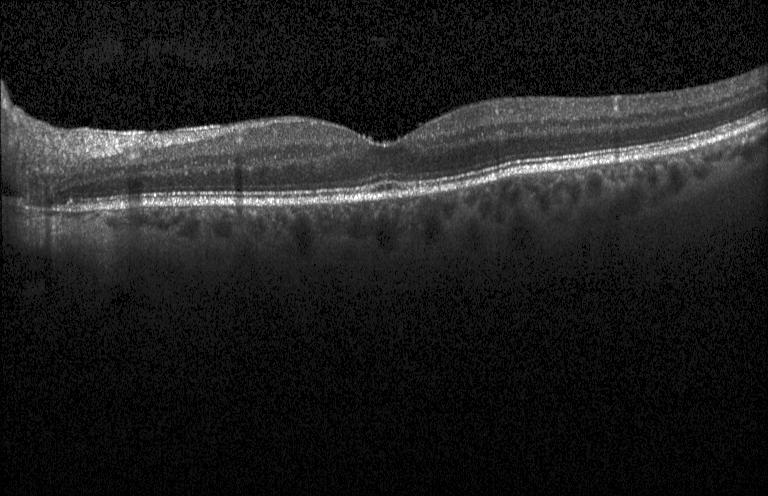

OCT B-scan; spectral-domain optical coherence tomography — No choroidal neovascularization, diabetic macular edema, or drusen.